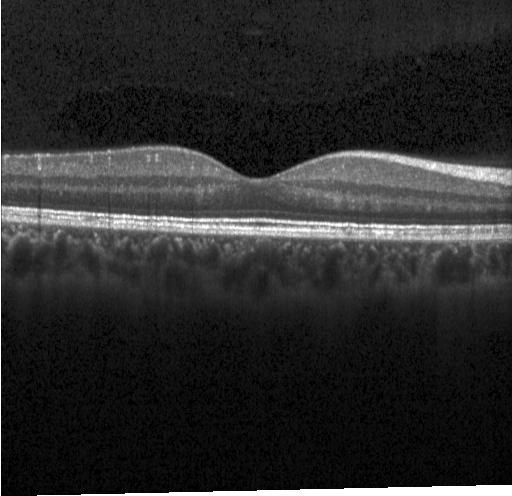

Retinal OCT cross-section, acquired on a Heidelberg Spectralis. Impression: neither CNV, DME, nor drusen.